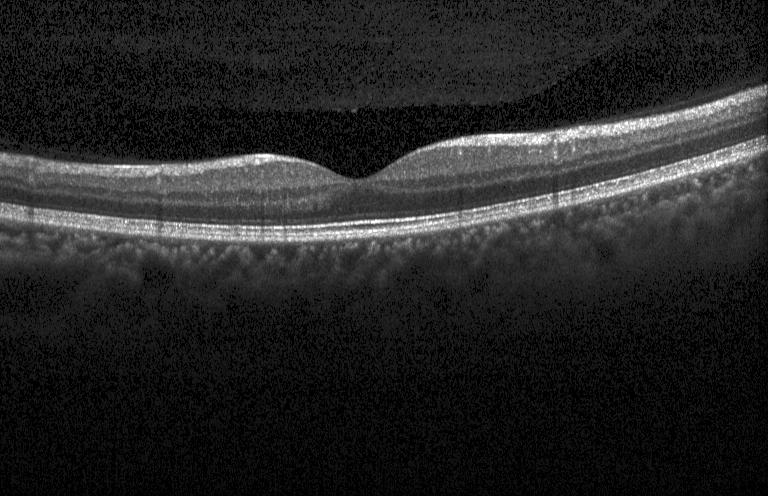 Diagnosis: no choroidal neovascularization, diabetic macular edema, or drusen.